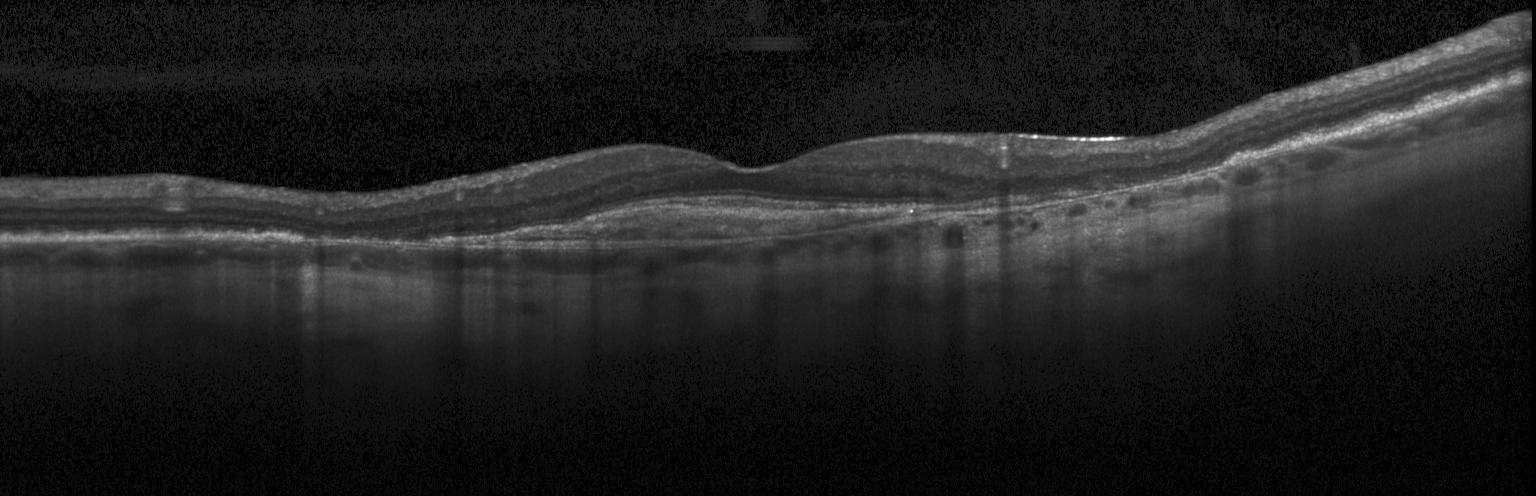
Finding: a choroidal neovascular membrane.